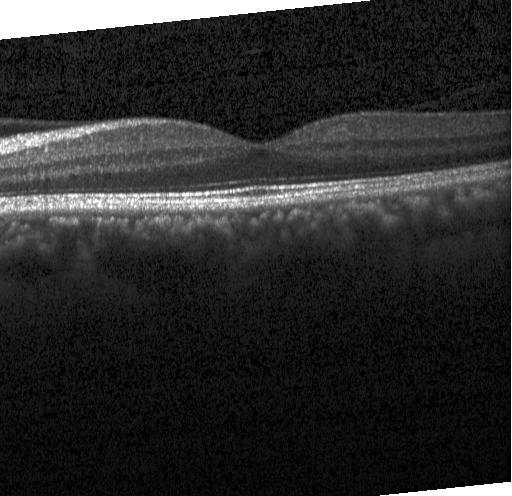

OCT line scan.
Finding: no choroidal neovascularization, diabetic macular edema, or drusen.